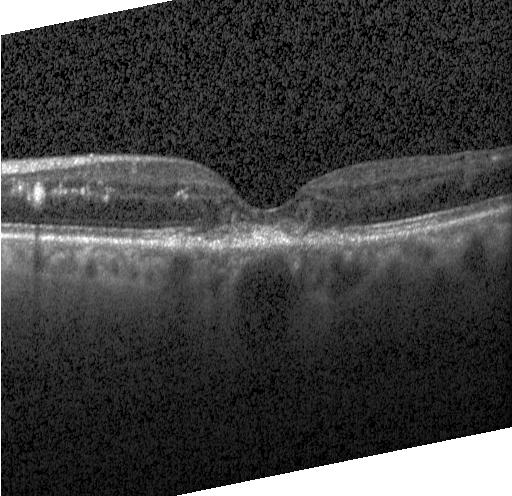 Retinal OCT cross-section
Impression: a choroidal neovascular membrane.